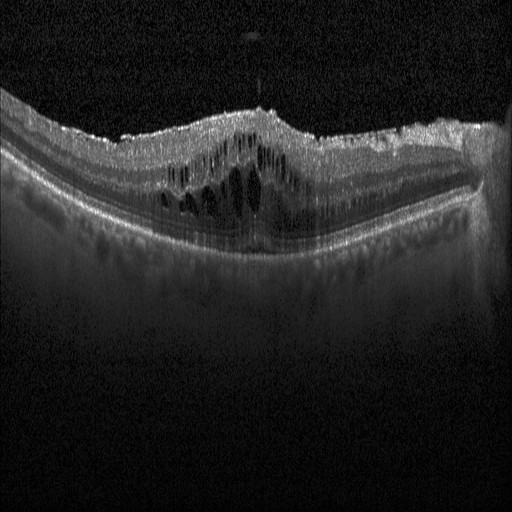
Diagnosis: diabetic macular edema.